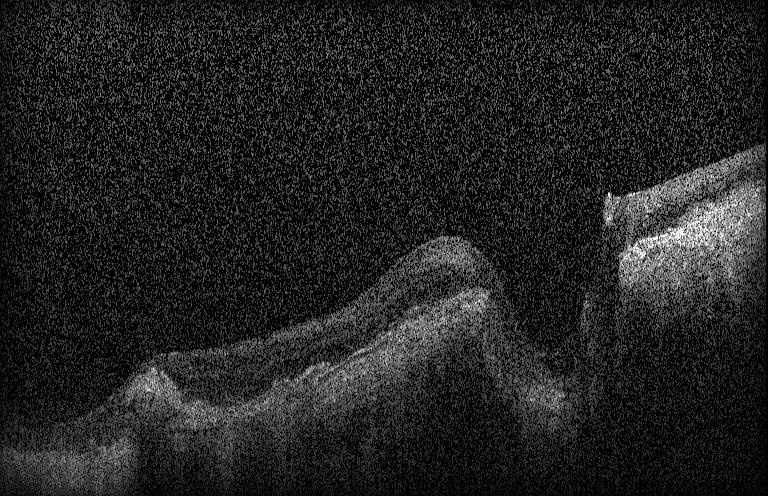
Retinal OCT B-scan.
Macular OCT: CNV.